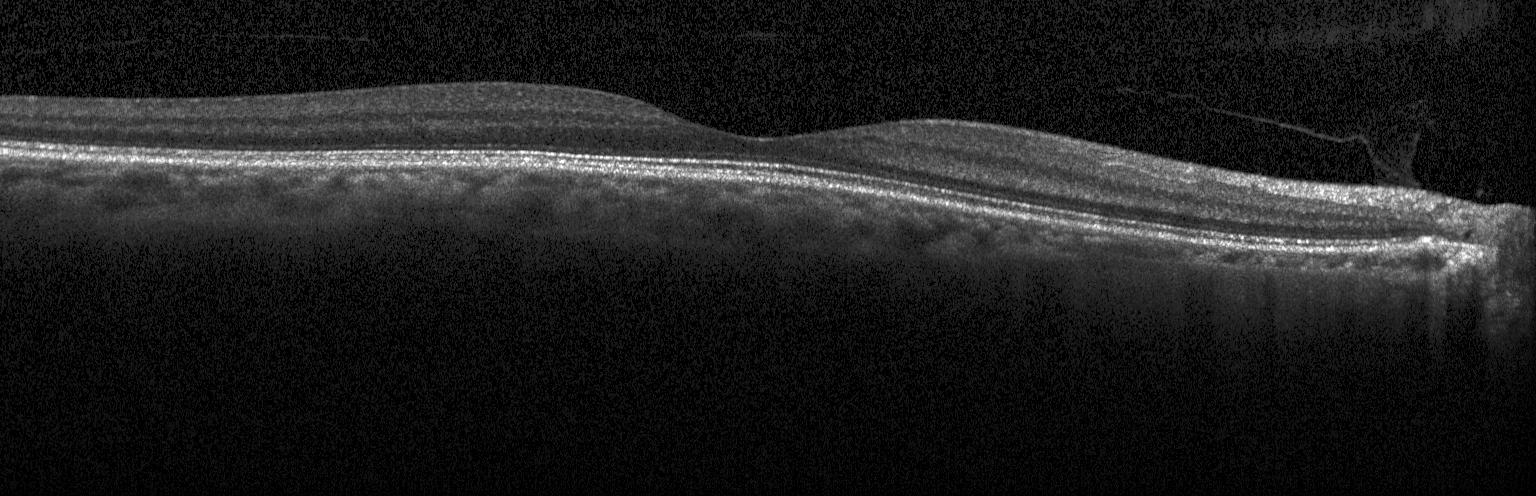 Spectral-domain optical coherence tomography; retinal OCT cross-section.
Diagnosis: no CNV, no DME, and no drusen.